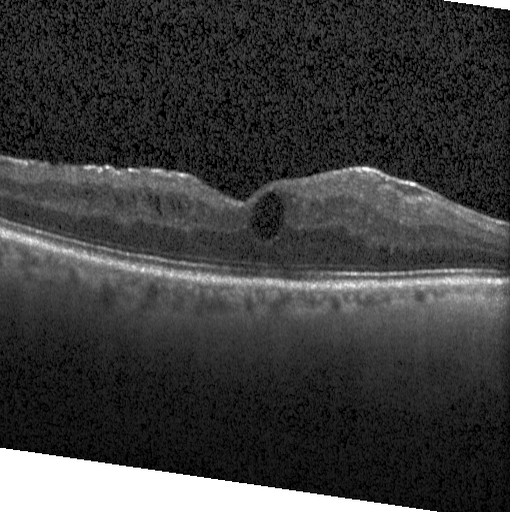

Macular scan · instrument: Heidelberg Spectralis · OCT line scan · spectral-domain OCT
Diagnosis: diabetic macular edema.